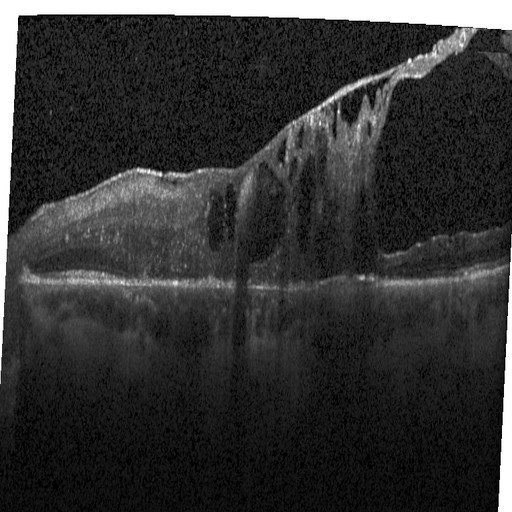 Dx: diabetic macular edema.